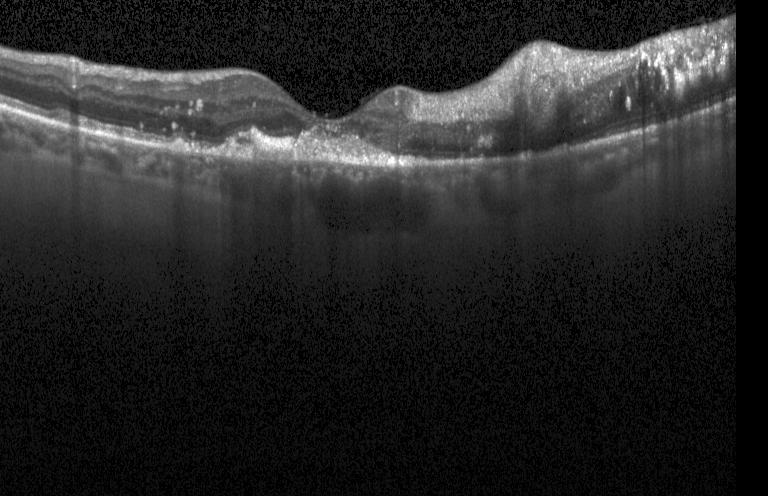

OCT line scan; spectral-domain OCT. Impression: a choroidal neovascular membrane.